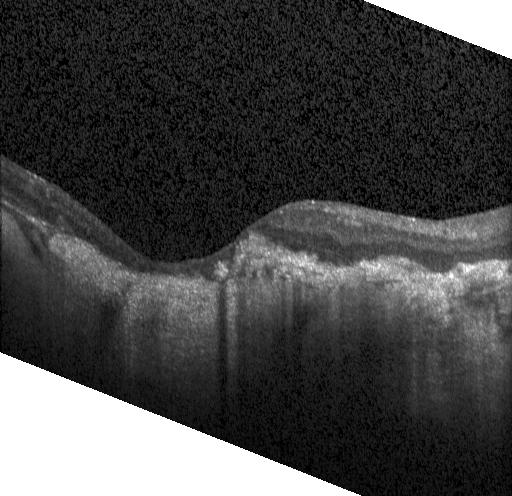
Finding: CNV.